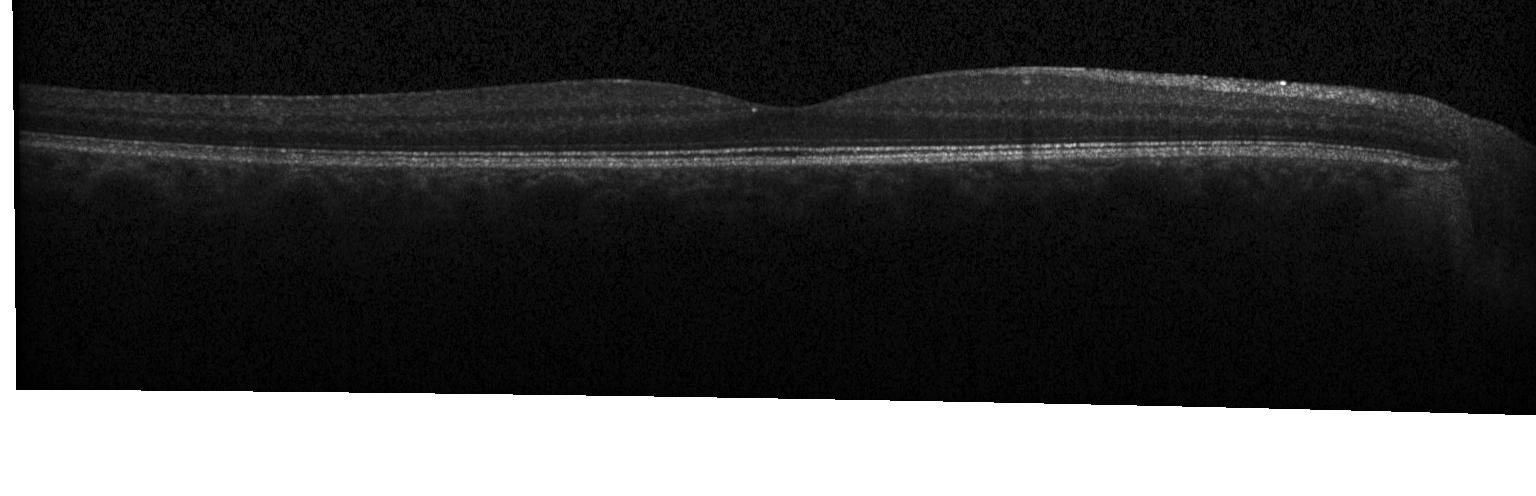

Impression: no evidence of CNV, DME, or drusen.